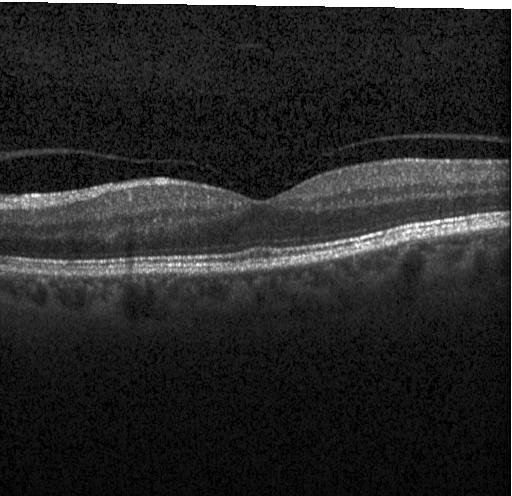
Impression: no CNV, DME, or drusen.